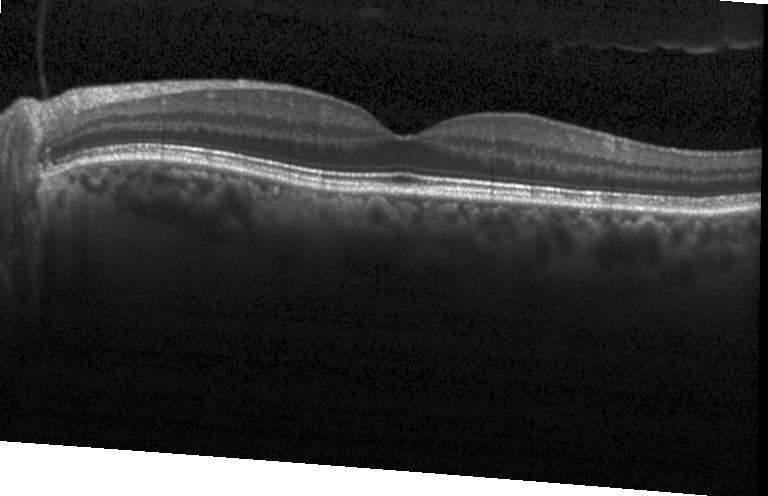

The scan shows no choroidal neovascularization, no diabetic macular edema, and no drusen.